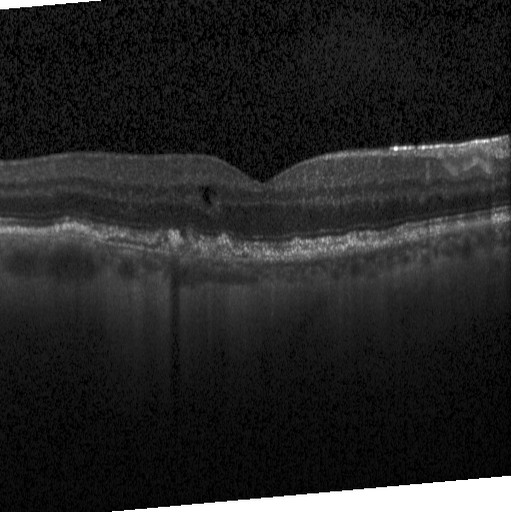

Assessment: diabetic macular edema.